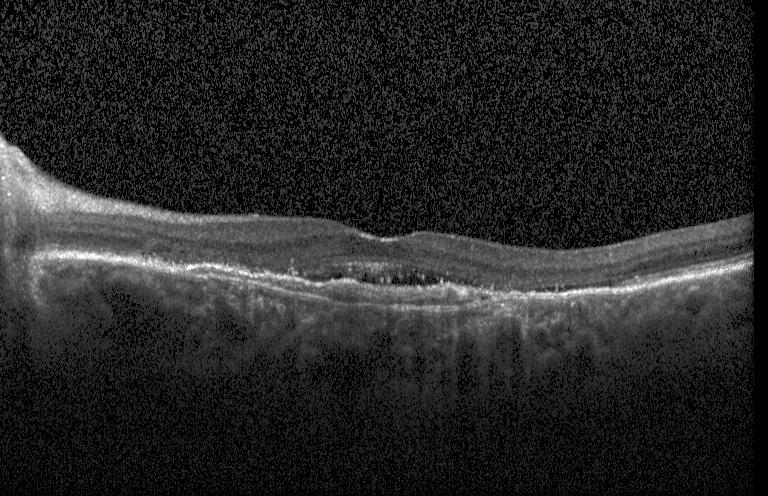 Retinal OCT cross-section showing a choroidal neovascular membrane.